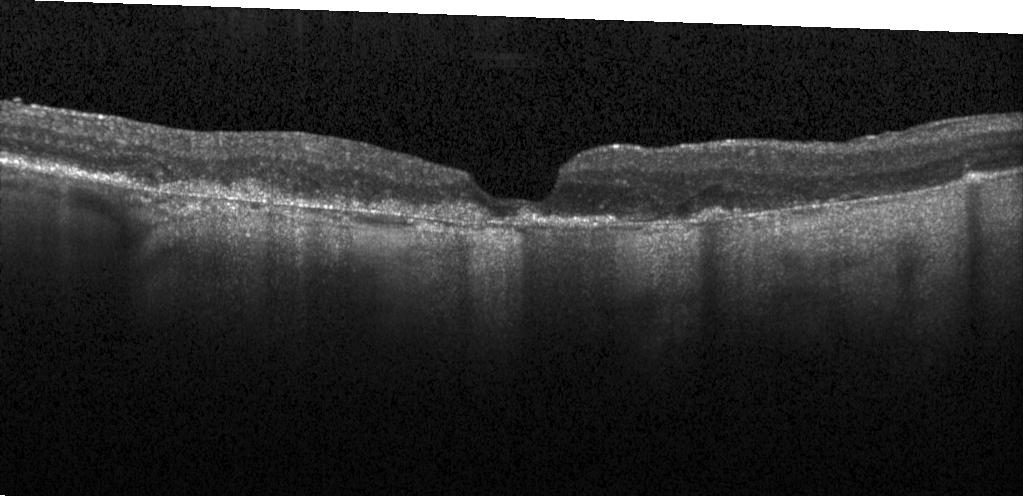

OCT line scan. Finding: a choroidal neovascular membrane.